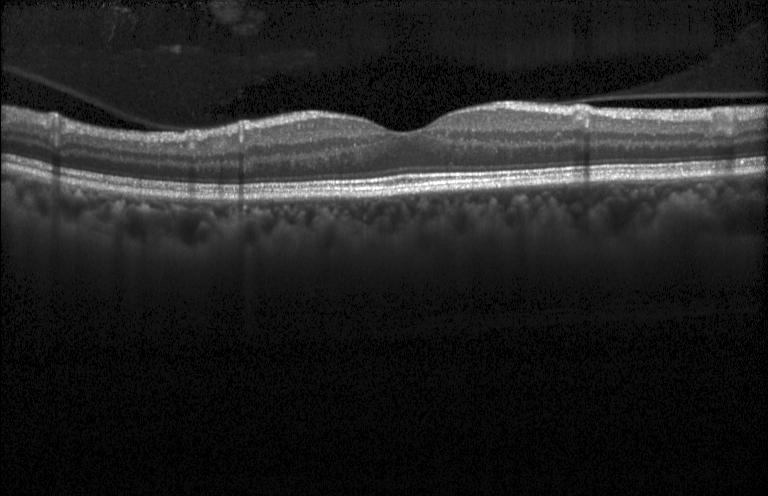 Impression: no evidence of CNV, DME, or drusen.